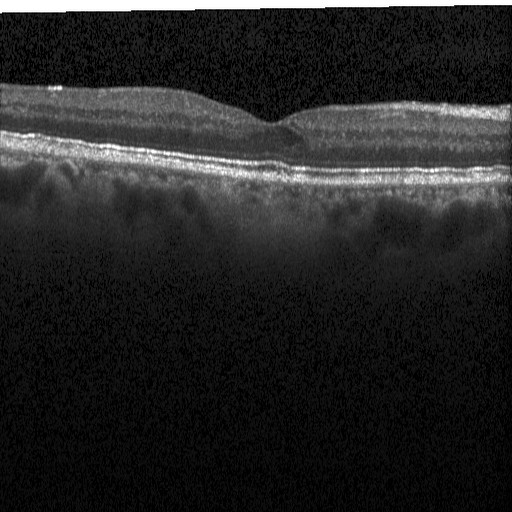
The scan shows DME.